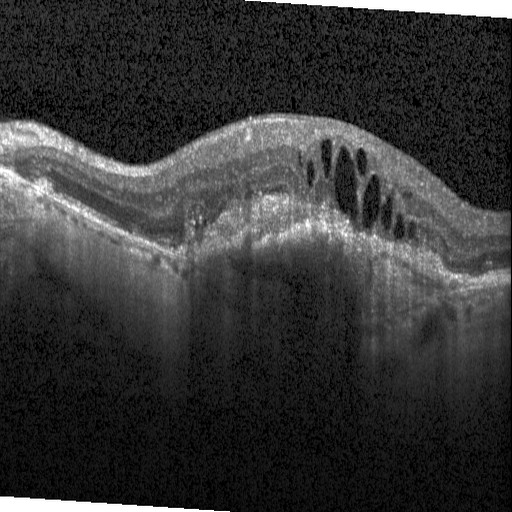

Impression: DME.